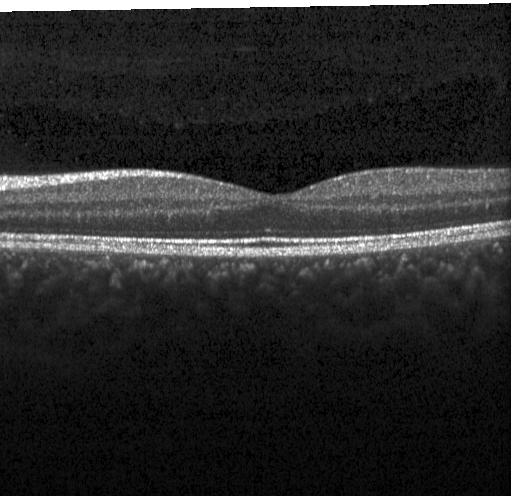

Diagnosis: no evidence of choroidal neovascularization, diabetic macular edema, or drusen.